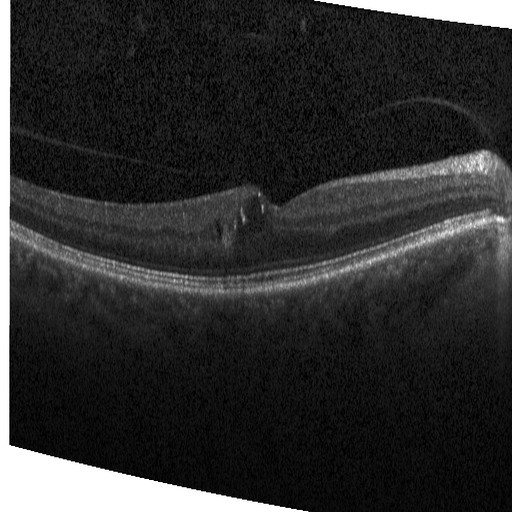 Finding: diabetic macular edema.